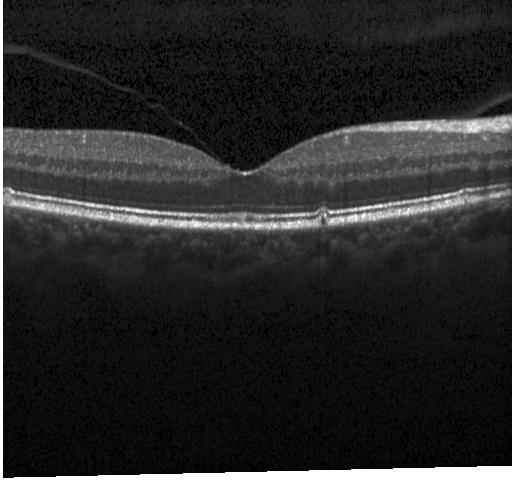

Optical coherence tomography scan · instrument: Heidelberg Spectralis
The scan shows multiple drusen.